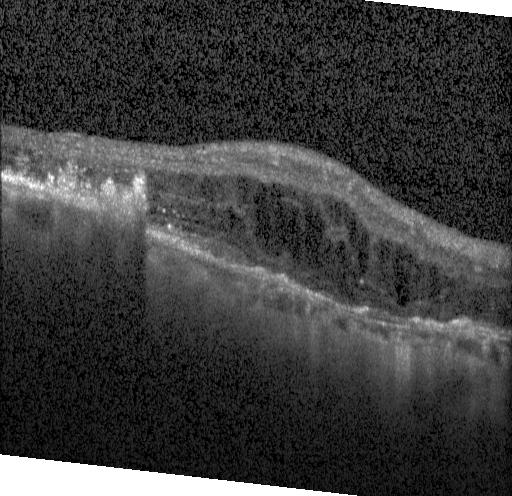 Spectral-domain optical coherence tomography; OCT B-scan; horizontal scan through the fovea.
Diagnosis: a choroidal neovascular membrane.